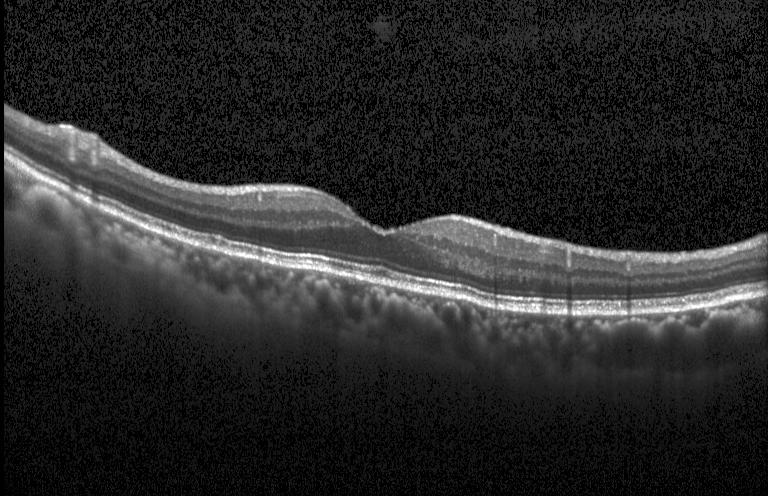
SD-OCT; OCT line scan; acquired on a Heidelberg Spectralis. Impression: neither CNV, DME, nor drusen.